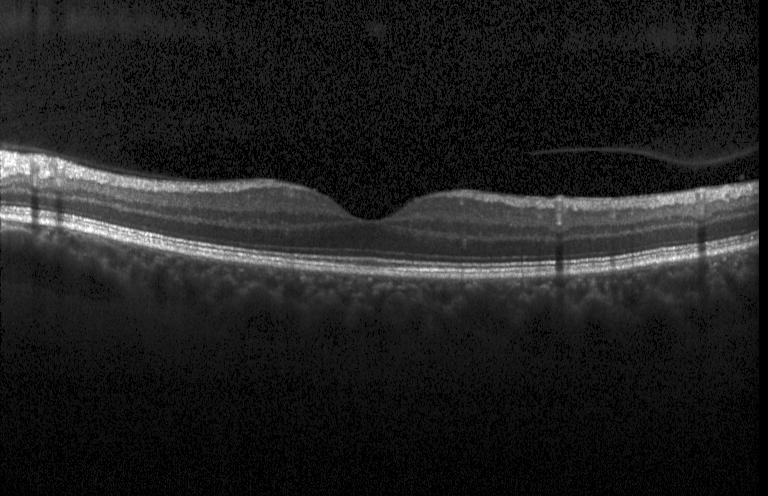 Impression: no choroidal neovascularization, no diabetic macular edema, and no drusen.